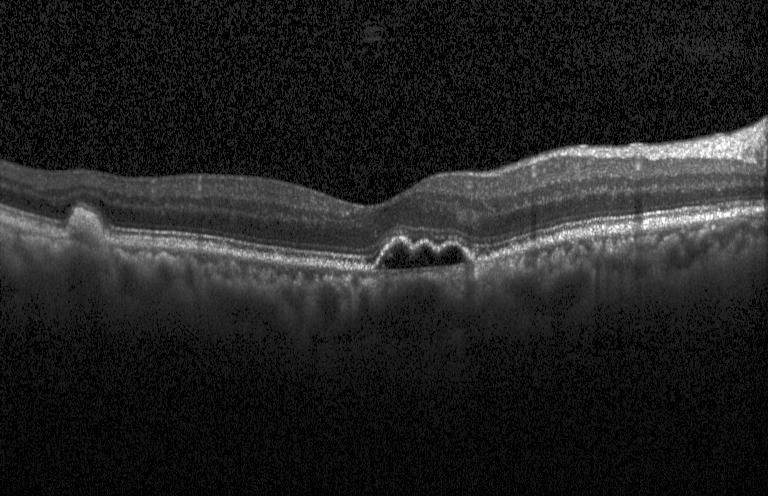

Choroidal neovascularization (CNV).